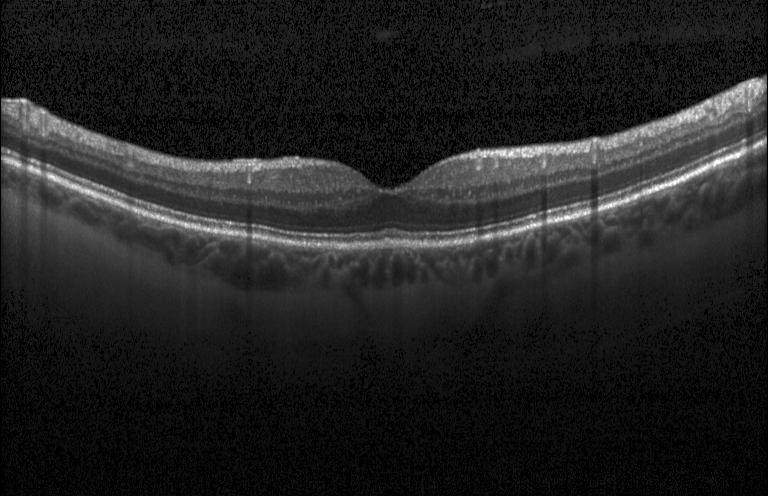 Diagnosis: no choroidal neovascularization, no diabetic macular edema, and no drusen.